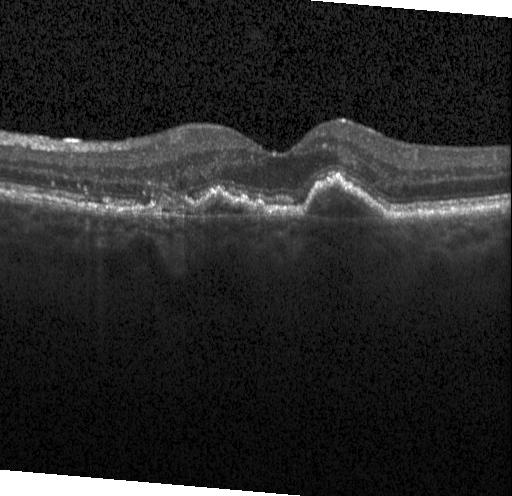 OCT line scan, spectral-domain OCT, macular scan. Assessment: choroidal neovascularization (CNV).